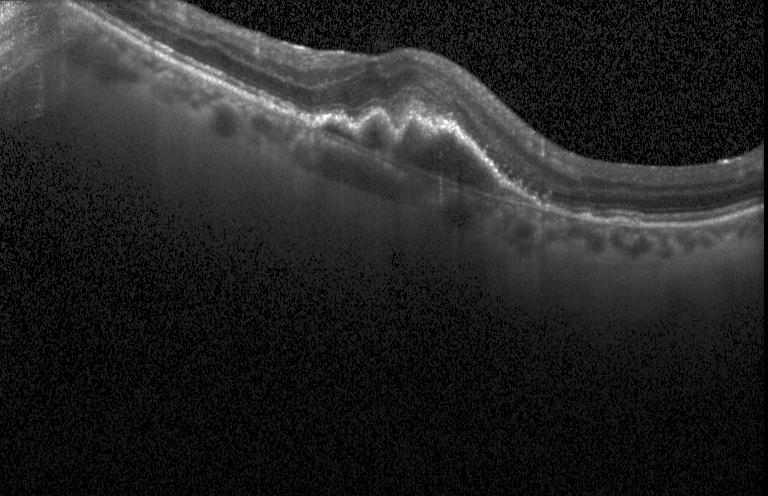 OCT B-scan. Instrument: Heidelberg Spectralis
Diagnosis: choroidal neovascularization.